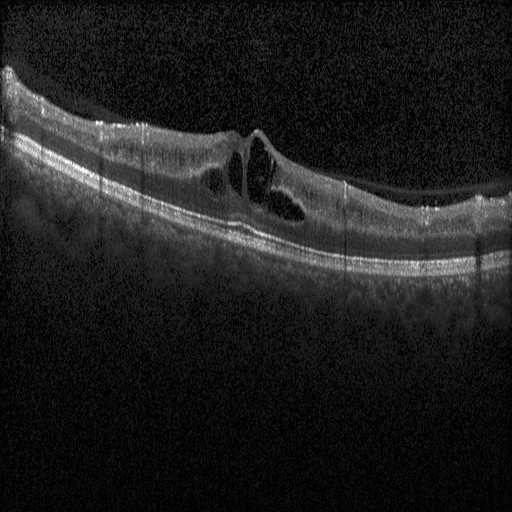
Macular OCT: diabetic macular edema (DME).